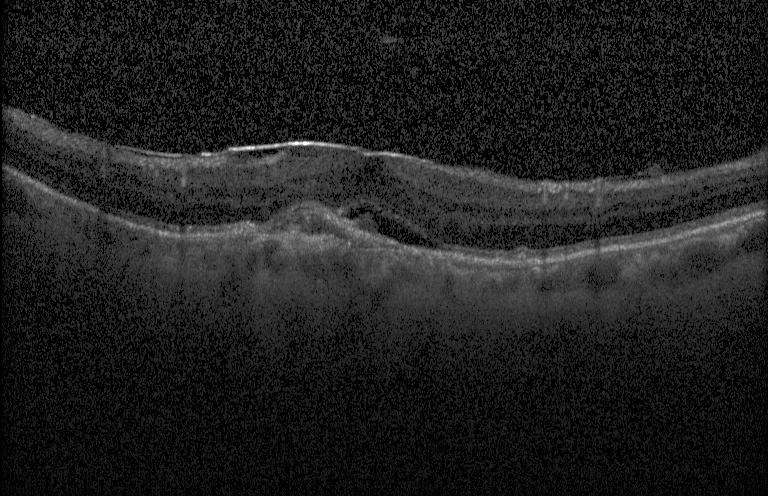

Dx: a choroidal neovascular membrane.